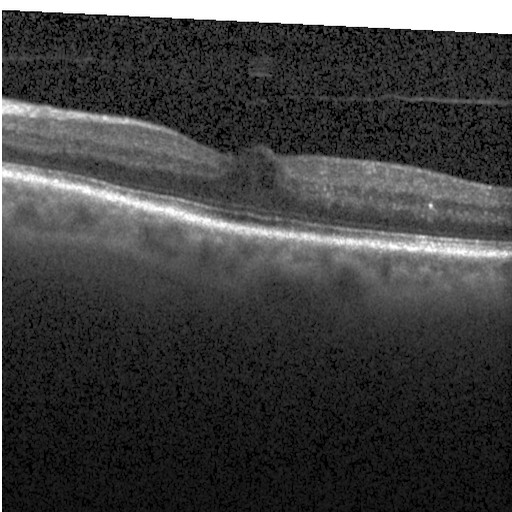
Diagnosis: diabetic macular edema (DME).